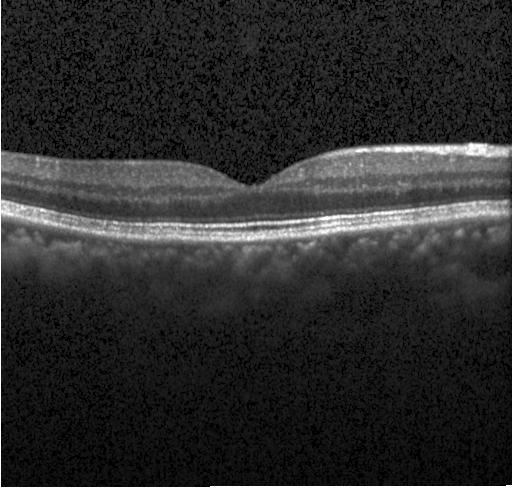
OCT B-scan. Heidelberg Spectralis OCT system. SD-OCT
Assessment: no evidence of CNV, DME, or drusen.